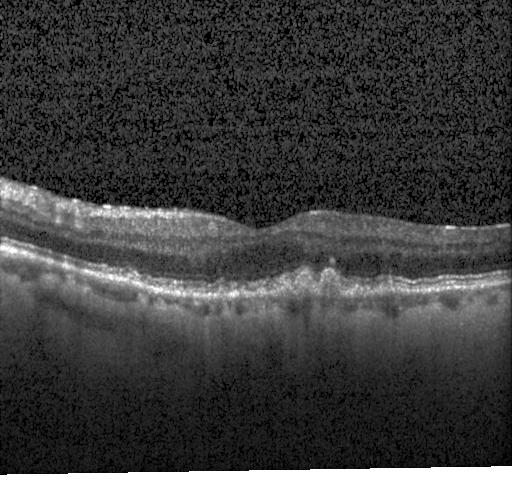 Macular OCT: drusen.